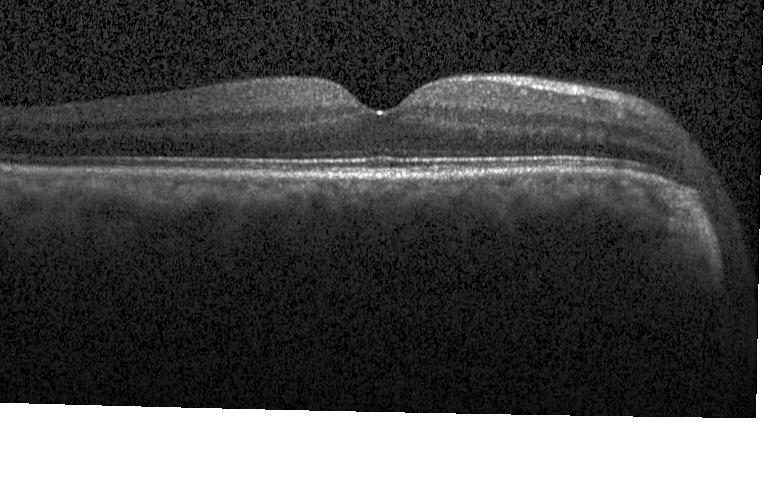 OCT line scan. Fovea-centered.
No choroidal neovascularization, diabetic macular edema, or drusen.